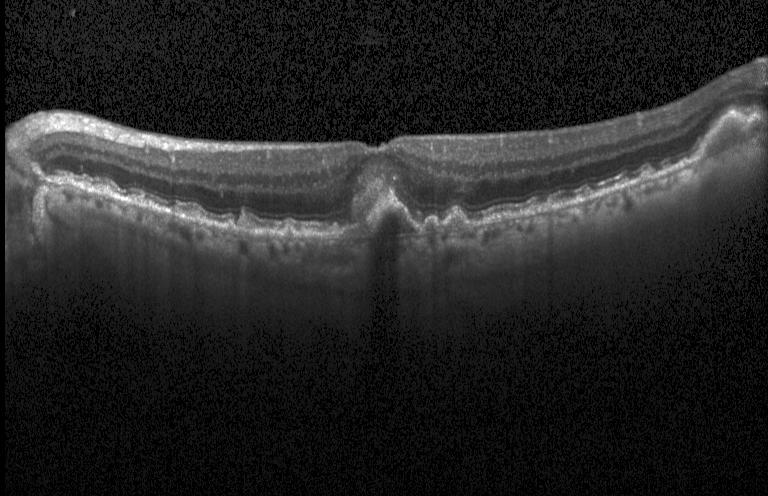

Spectral-domain optical coherence tomography. Macular scan. OCT line scan
Diagnosis: choroidal neovascularization (CNV).